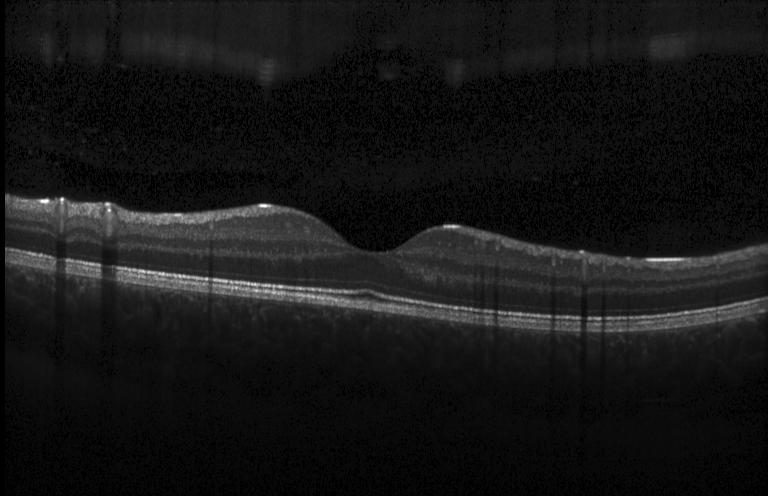
Finding: no choroidal neovascularization, diabetic macular edema, or drusen.